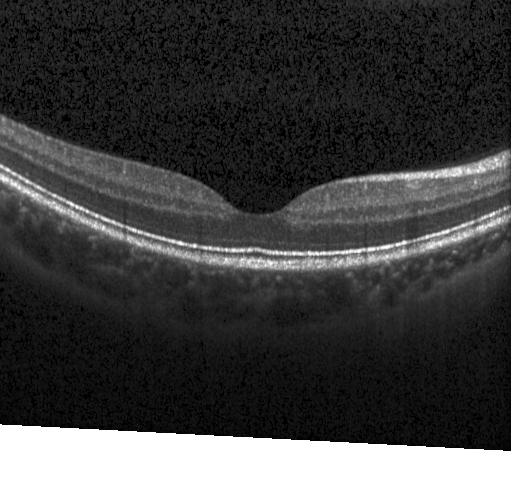 This B-scan demonstrates no CNV, DME, or drusen.